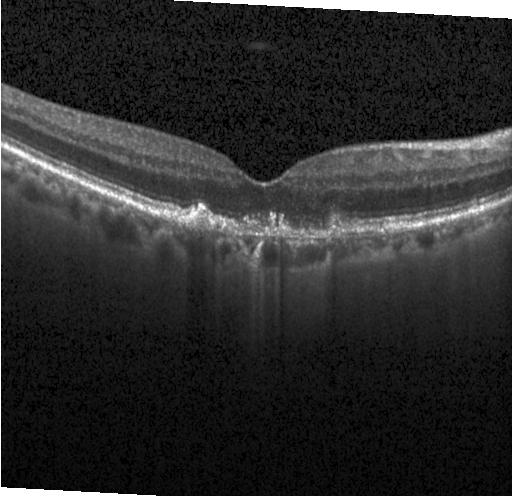

Retinal OCT B-scan; horizontal scan through the fovea; acquired on a Heidelberg Spectralis; spectral-domain OCT
This B-scan demonstrates drusen.